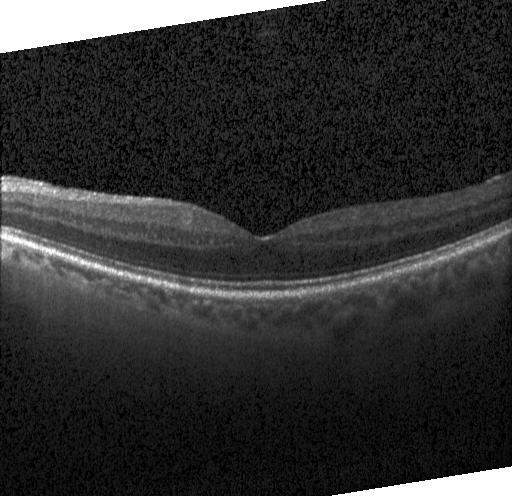

Impression: no evidence of CNV, DME, or drusen.